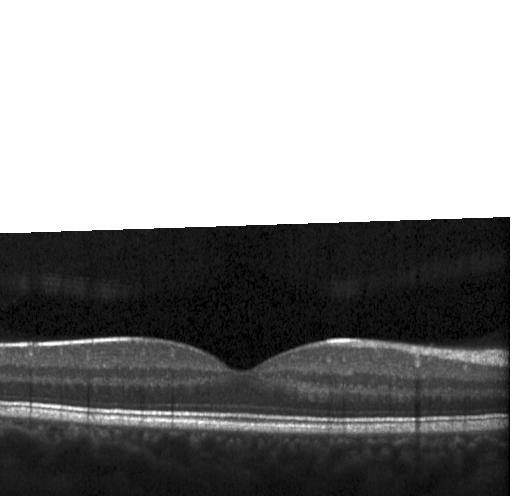 Optical coherence tomography scan, through the macula, spectral-domain OCT, Heidelberg Spectralis OCT system.
No CNV, no DME, and no drusen.